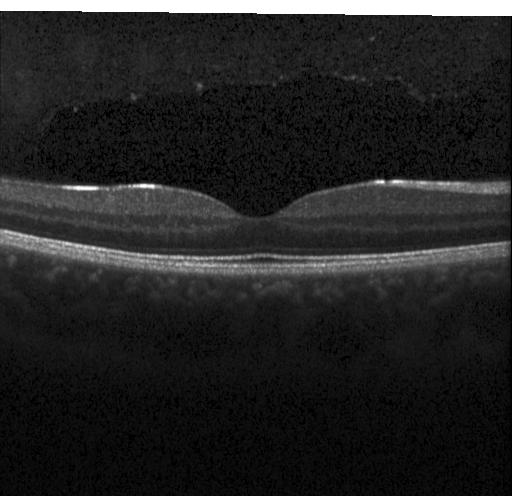
OCT line scan — Finding: no choroidal neovascularization, diabetic macular edema, or drusen.